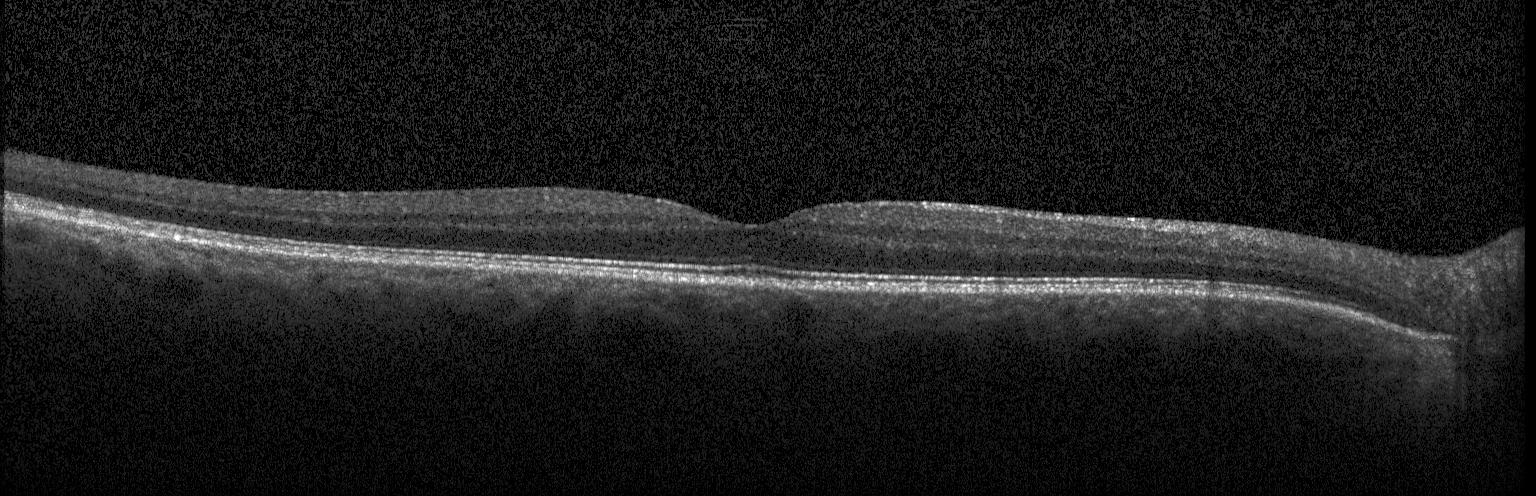 Diagnosis: neither CNV, DME, nor drusen.